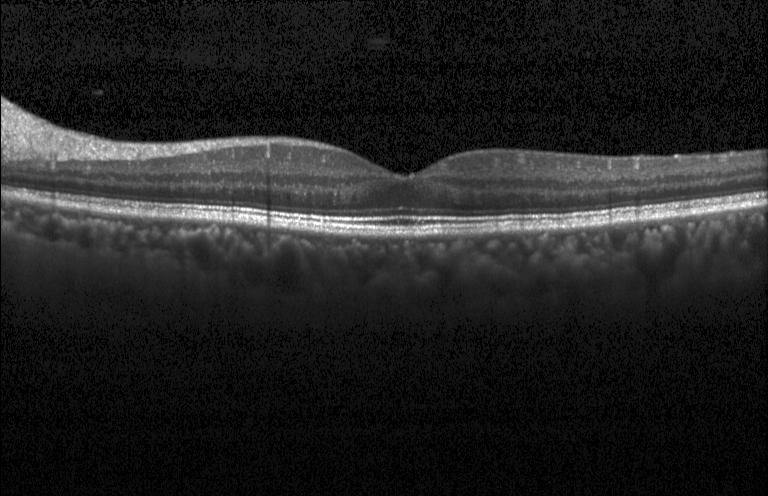
Retinal OCT B-scan. OCT finding: neither CNV, DME, nor drusen.